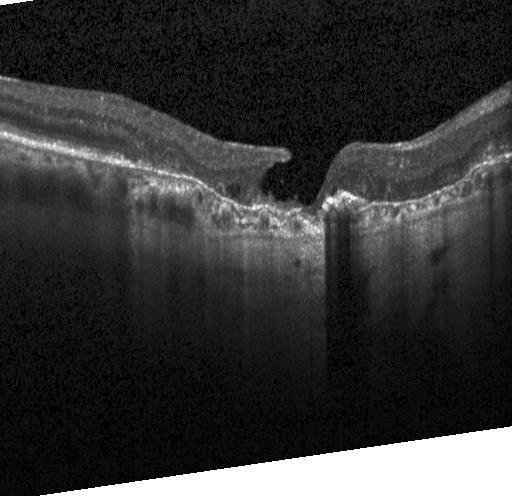 Diagnosis: CNV.